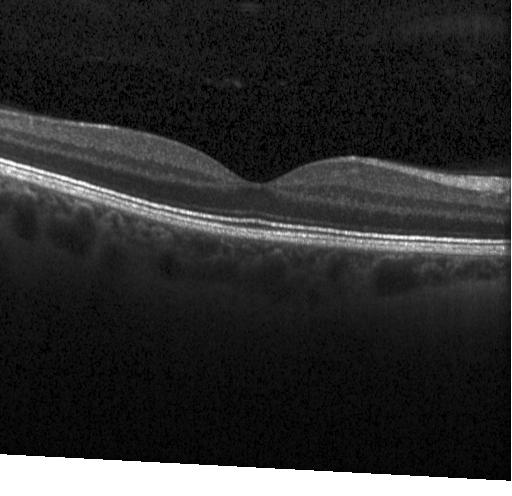 Retinal OCT cross-section, centered on the fovea, acquired on a Heidelberg Spectralis
Diagnosis: no CNV, DME, or drusen.